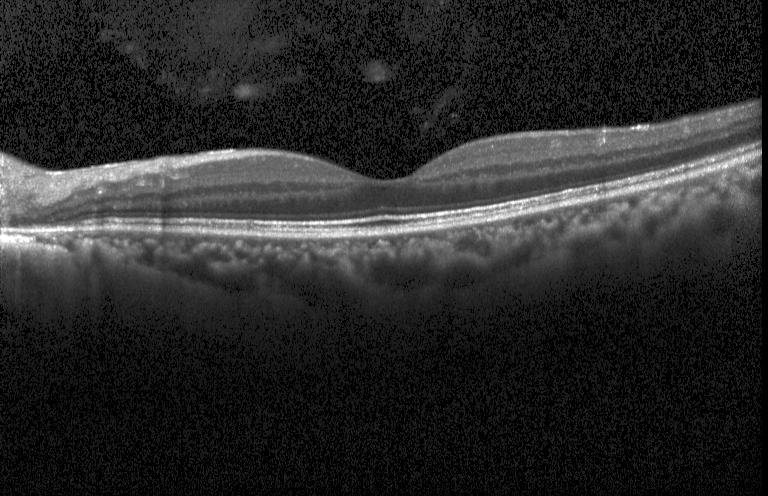 Optical coherence tomography scan, spectral-domain optical coherence tomography, horizontal scan through the fovea. Finding: no evidence of choroidal neovascularization, diabetic macular edema, or drusen.